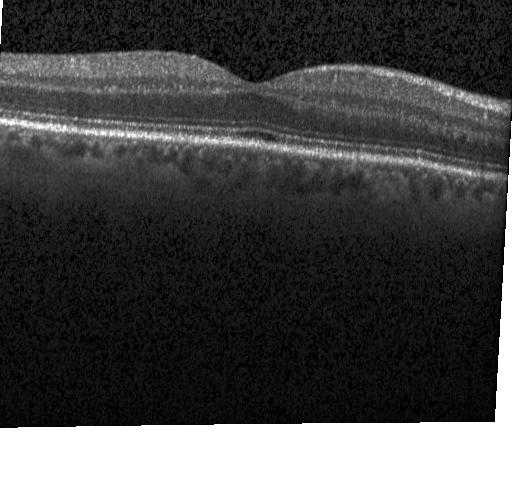
Retinal OCT cross-section.
Diagnosis: no choroidal neovascularization, diabetic macular edema, or drusen.